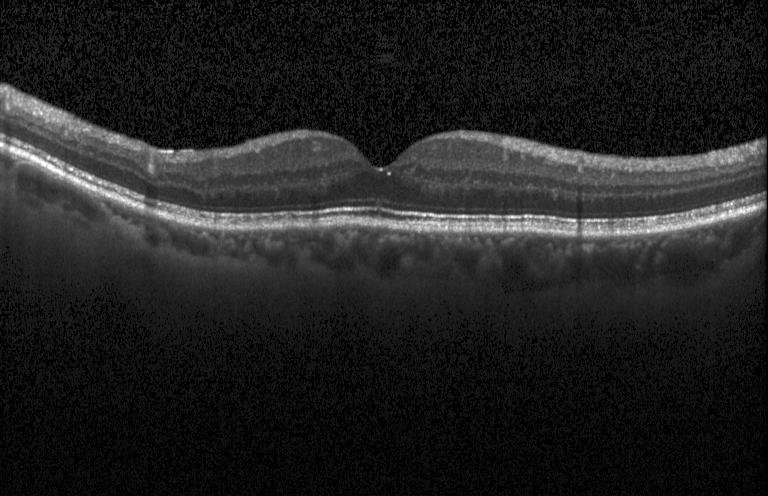
Horizontal scan through the fovea · optical coherence tomography B-scan.
Macular OCT: no evidence of choroidal neovascularization, diabetic macular edema, or drusen.